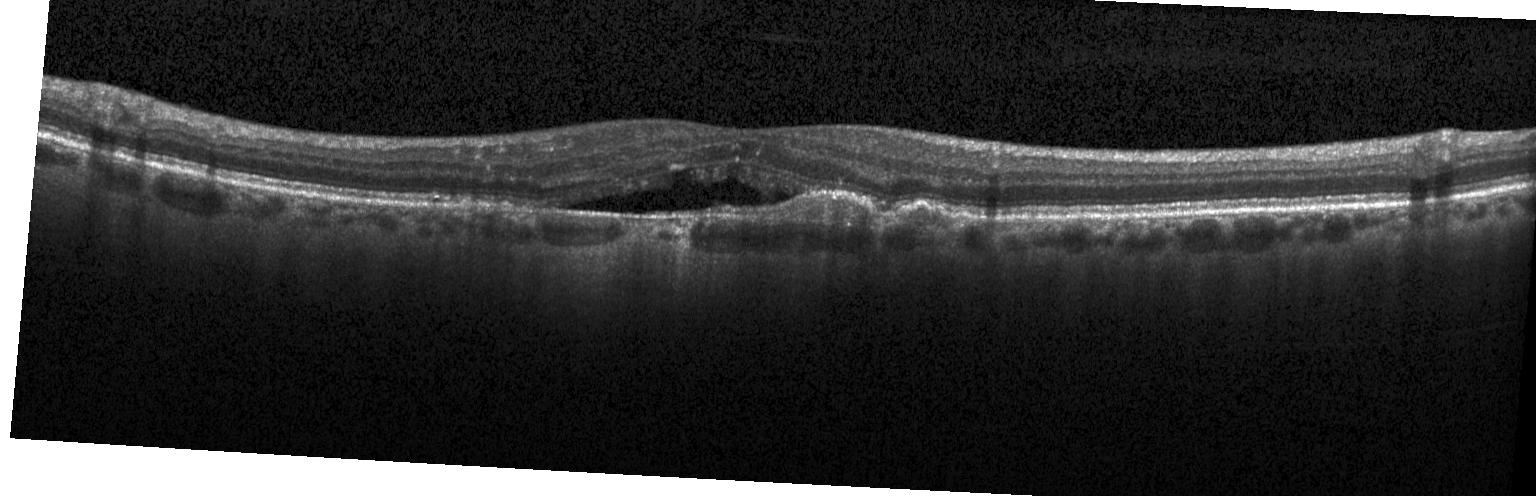

Spectral-domain optical coherence tomography; retinal OCT cross-section
Finding: choroidal neovascularization (CNV).